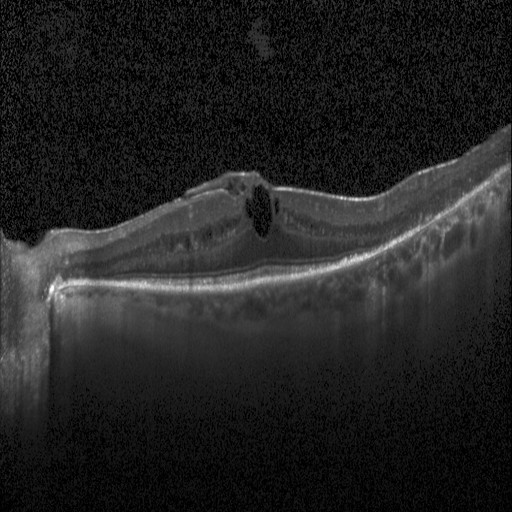
The scan shows diabetic macular edema.